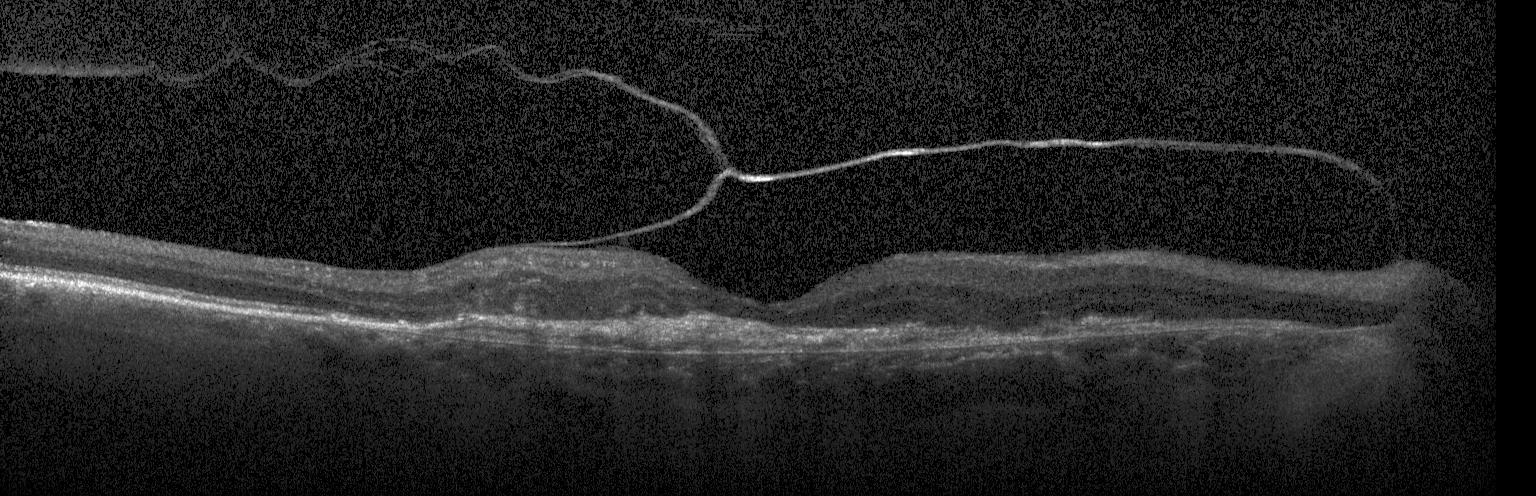
OCT B-scan, fovea-centered, spectral-domain OCT.
Impression: choroidal neovascularization (CNV).